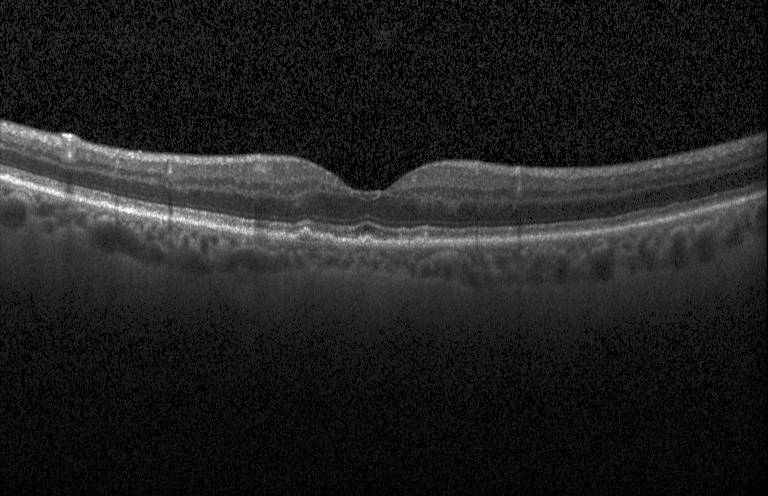
Macular OCT: sub-RPE drusenoid deposits.